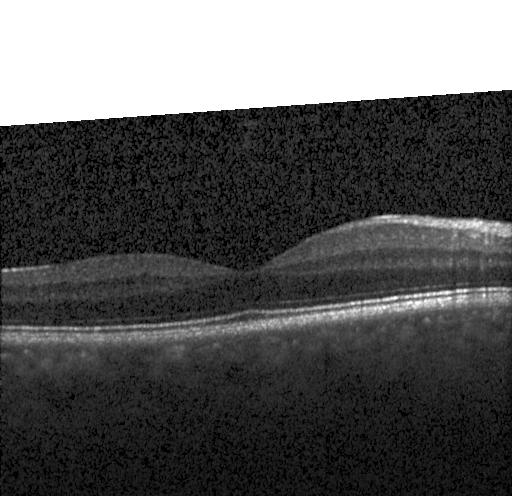
Instrument: Heidelberg Spectralis; retinal OCT cross-section; macular scan; spectral-domain OCT — OCT finding: no evidence of choroidal neovascularization, diabetic macular edema, or drusen.